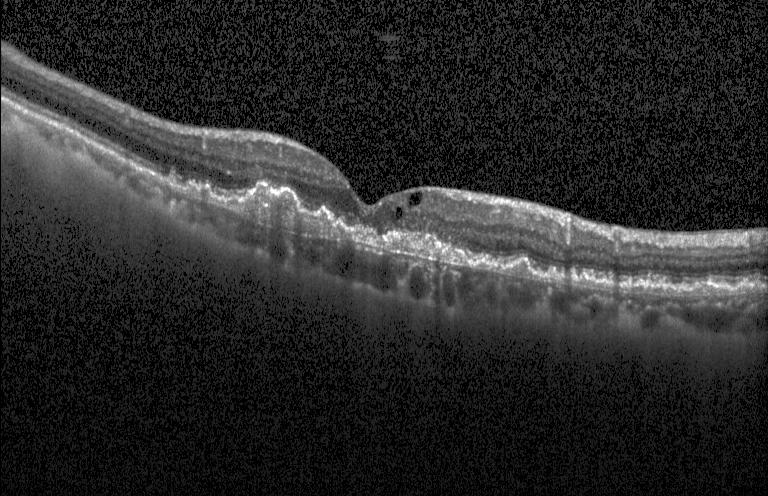

Macular scan. Optical coherence tomography B-scan. Instrument: Heidelberg Spectralis.
Dx: CNV.